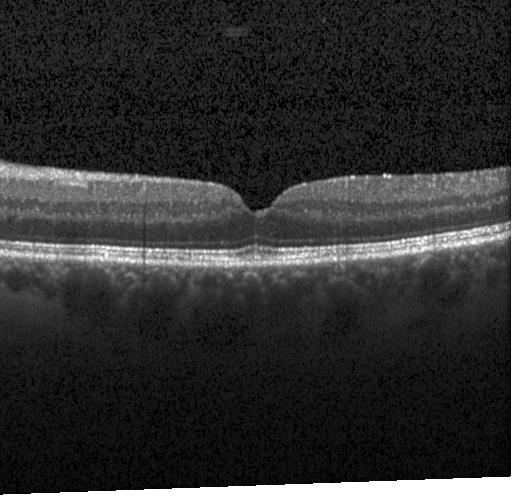

Assessment: no choroidal neovascularization, no diabetic macular edema, and no drusen.